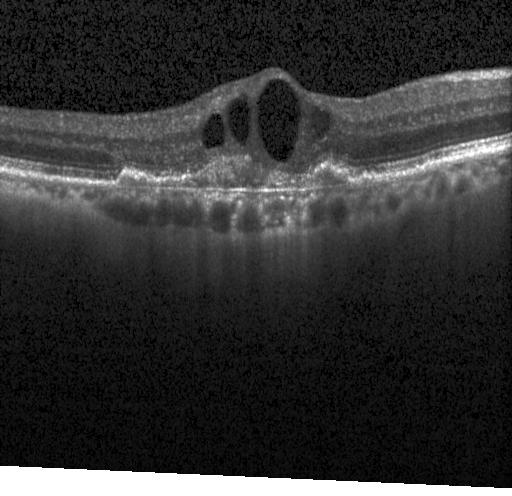 Heidelberg Spectralis; OCT B-scan; SD-OCT. This B-scan demonstrates a choroidal neovascular membrane.